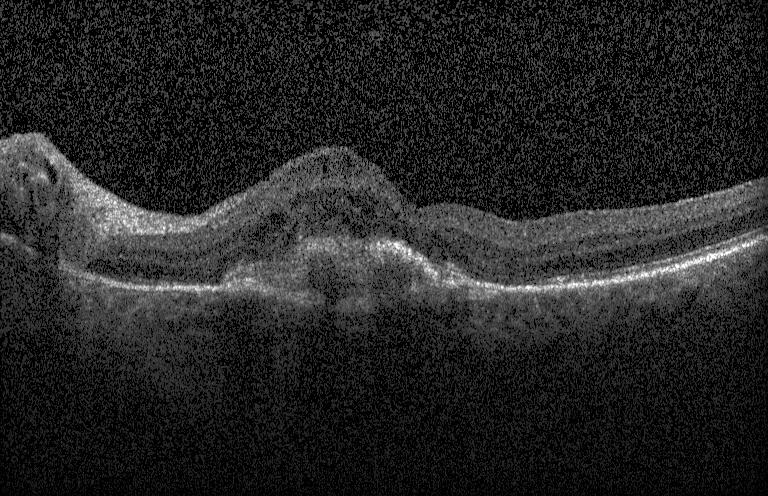

Retinal OCT B-scan; spectral-domain optical coherence tomography; instrument: Heidelberg Spectralis
The scan shows CNV.